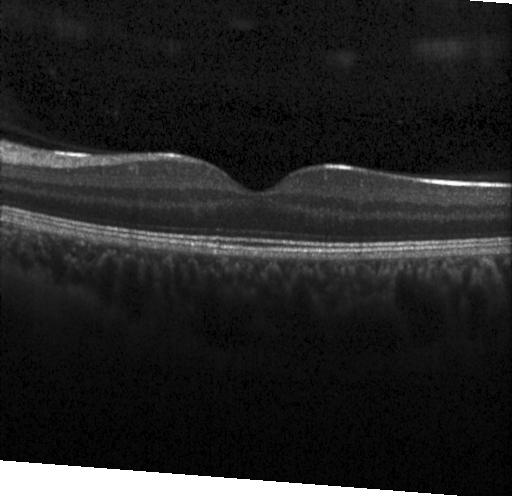
Heidelberg Spectralis OCT system · spectral-domain optical coherence tomography · retinal OCT cross-section · macular scan. Macular OCT: no CNV, DME, or drusen.